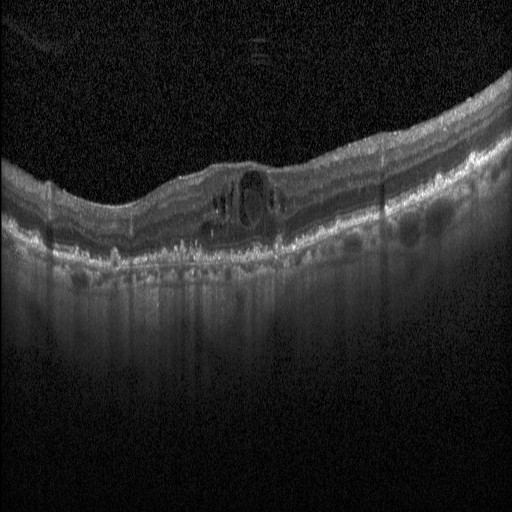 Assessment: diabetic macular edema (DME).